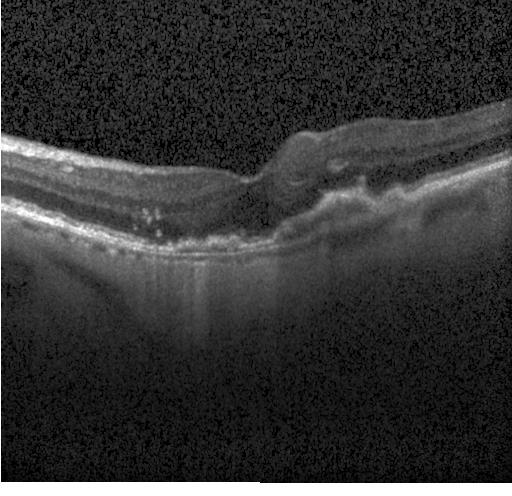

OCT line scan.
Diagnosis: choroidal neovascularization.